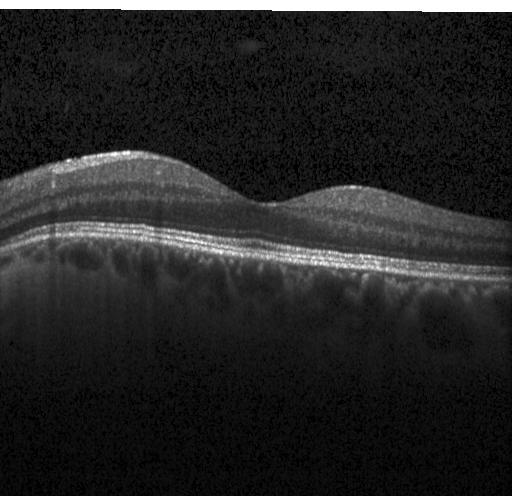 Acquired on a Heidelberg Spectralis. Centered on the fovea. SD-OCT. Optical coherence tomography scan. Finding: no evidence of choroidal neovascularization, diabetic macular edema, or drusen.